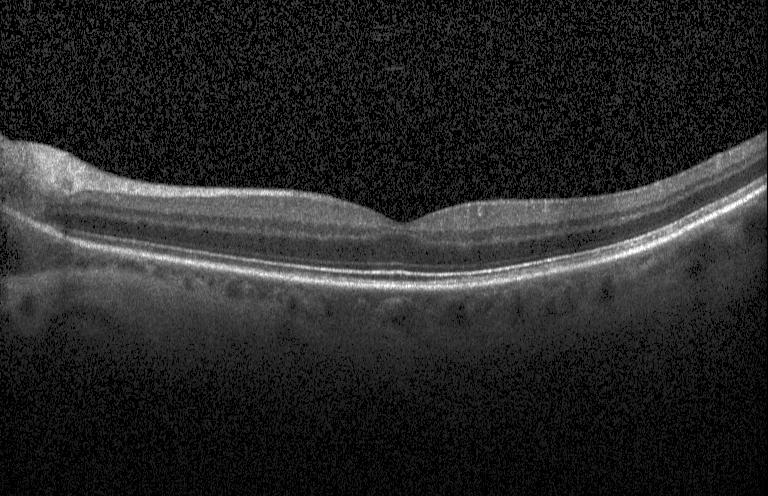

Instrument: Heidelberg Spectralis. Retinal OCT B-scan. Spectral-domain optical coherence tomography. Centered on the fovea. Finding: no choroidal neovascularization, no diabetic macular edema, and no drusen.